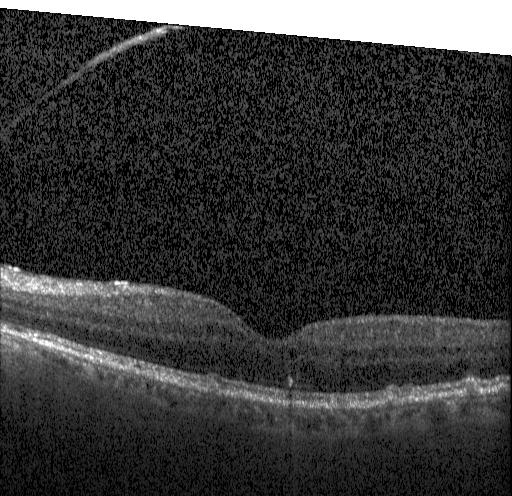 Through the macula; retinal OCT cross-section.
The scan shows multiple drusen.